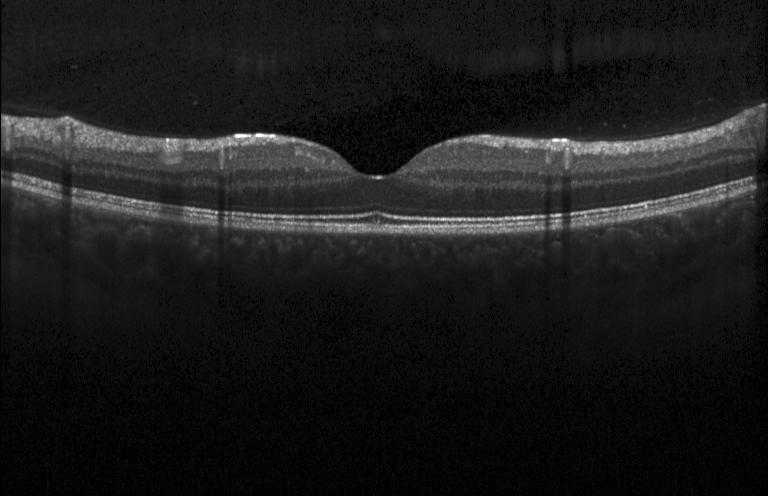

Diagnosis: no evidence of CNV, DME, or drusen.